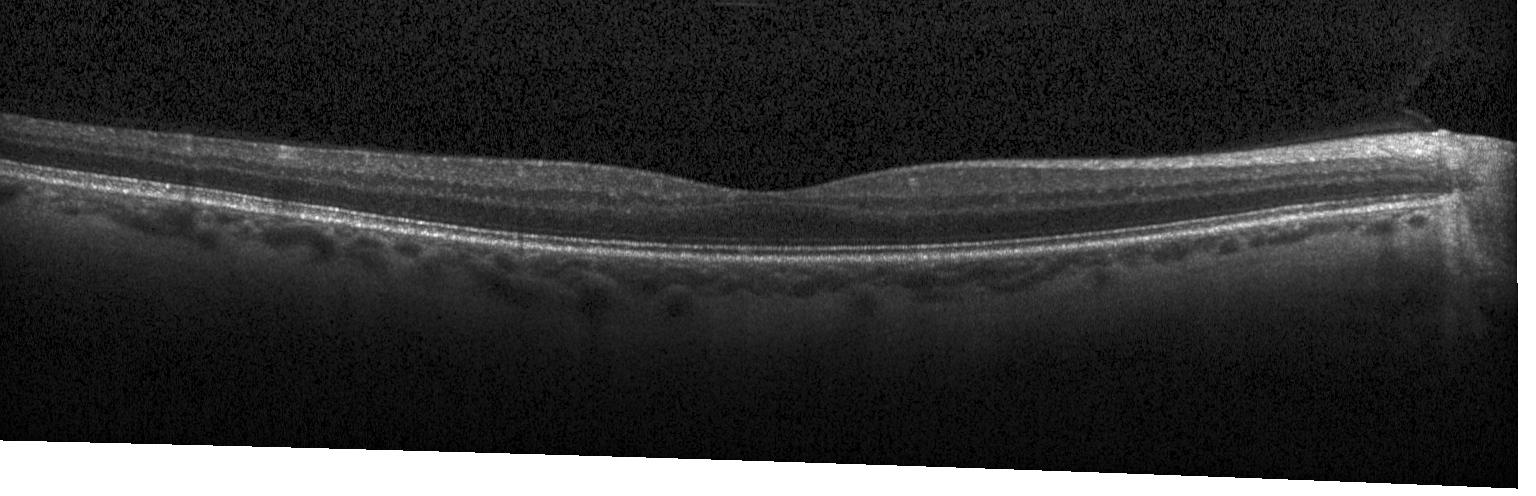

SD-OCT. Instrument: Heidelberg Spectralis. OCT B-scan. Fovea-centered
Dx: neither choroidal neovascularization, diabetic macular edema, nor drusen.